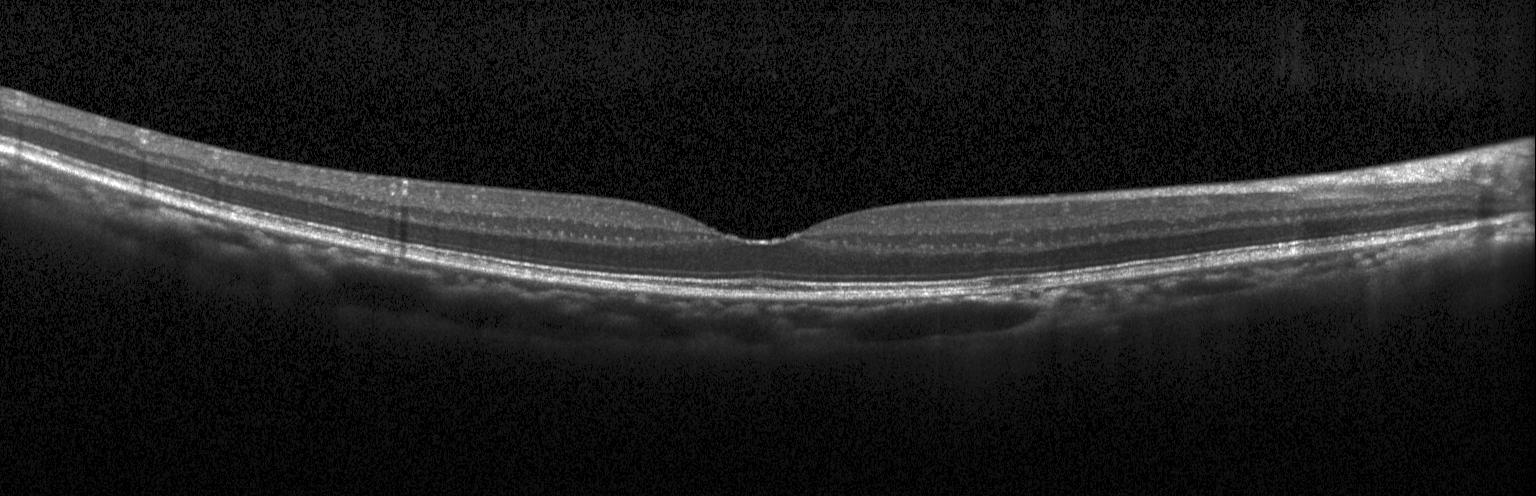
Instrument: Heidelberg Spectralis · retinal OCT cross-section.
This B-scan demonstrates no evidence of choroidal neovascularization, diabetic macular edema, or drusen.